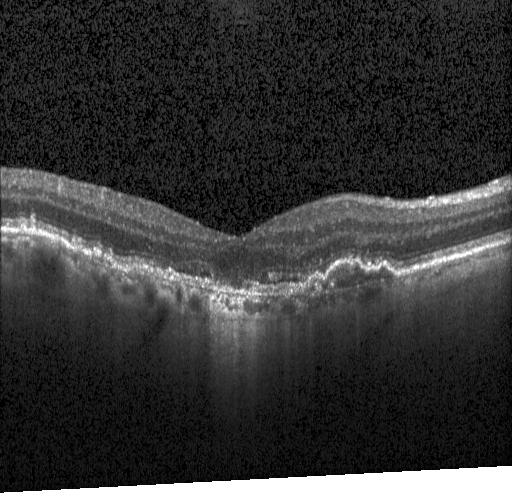 Dx: a choroidal neovascular membrane.